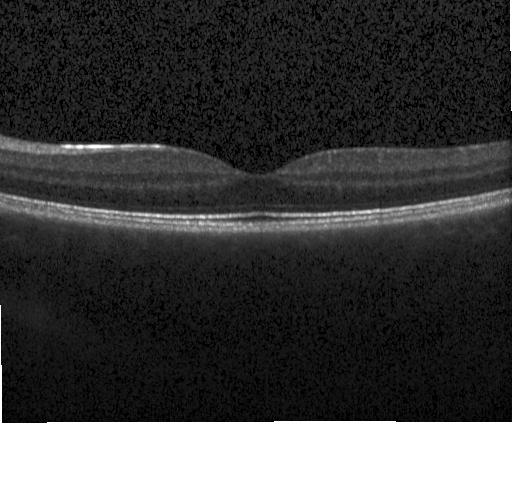
Optical coherence tomography B-scan; through the macula; spectral-domain optical coherence tomography; Heidelberg Spectralis.
The scan shows no choroidal neovascularization, no diabetic macular edema, and no drusen.